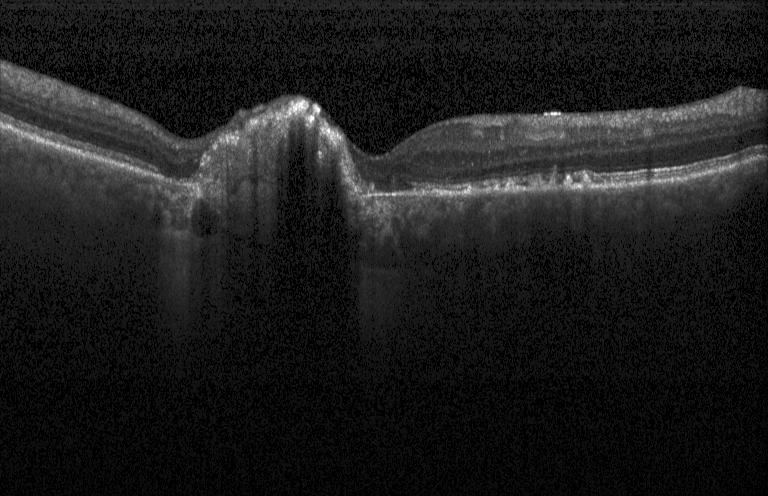 Optical coherence tomography B-scan · Heidelberg Spectralis · spectral-domain optical coherence tomography
OCT finding: a choroidal neovascular membrane.